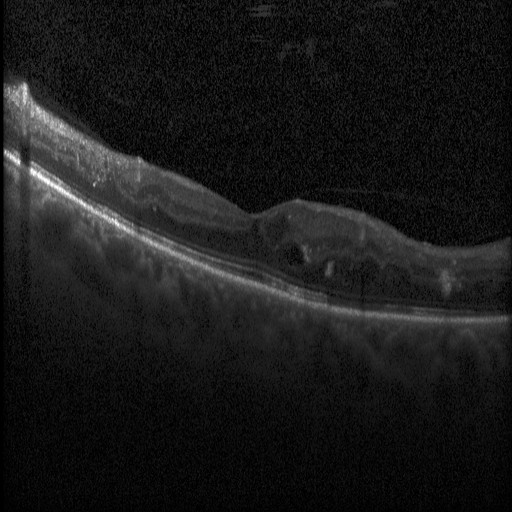
Spectral-domain OCT B-scan: diabetic macular edema.